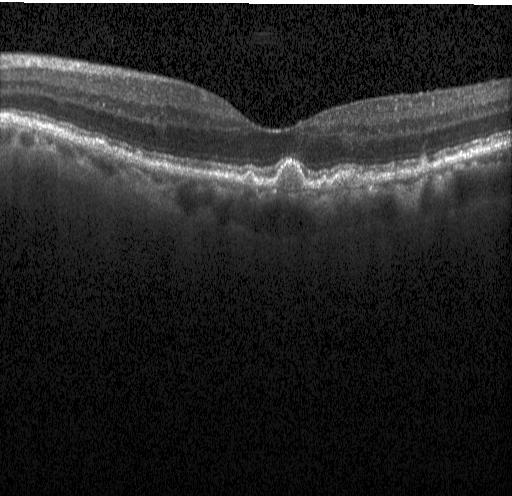

Retinal OCT B-scan, horizontal scan through the fovea, SD-OCT, Heidelberg Spectralis. Finding: multiple drusen.